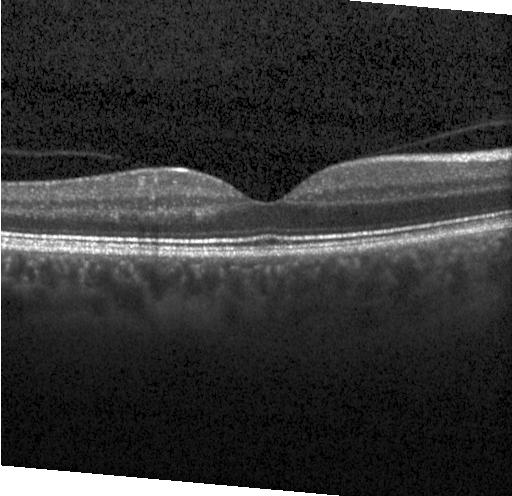

Optical coherence tomography B-scan. Through the macula. Spectral-domain OCT. Heidelberg Spectralis
Finding: neither choroidal neovascularization, diabetic macular edema, nor drusen.